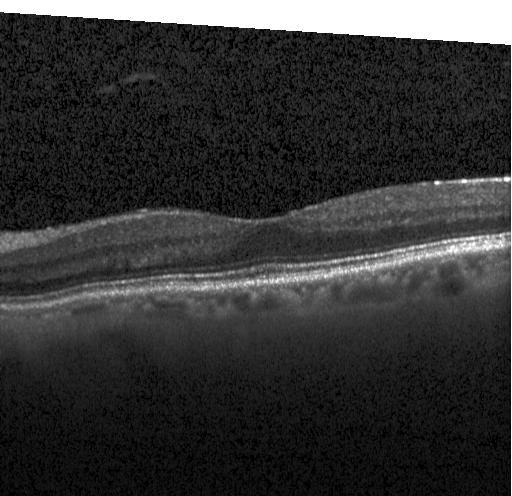
Retinal OCT B-scan. Diagnosis: no choroidal neovascularization, diabetic macular edema, or drusen.